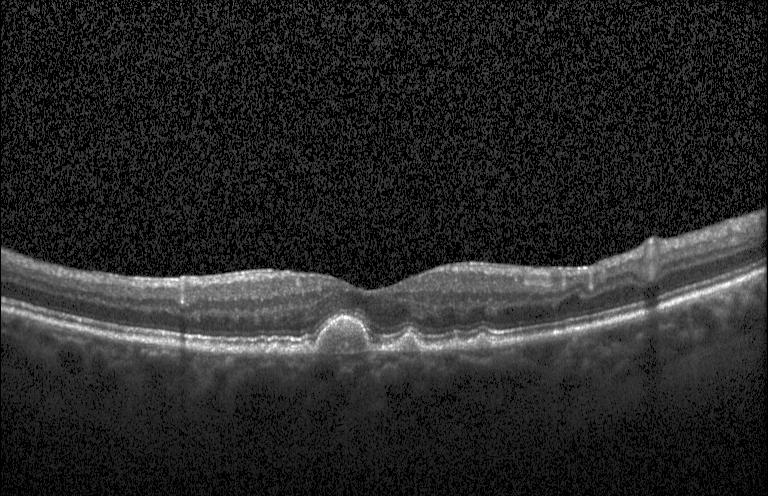
Macular OCT: sub-RPE drusenoid deposits.